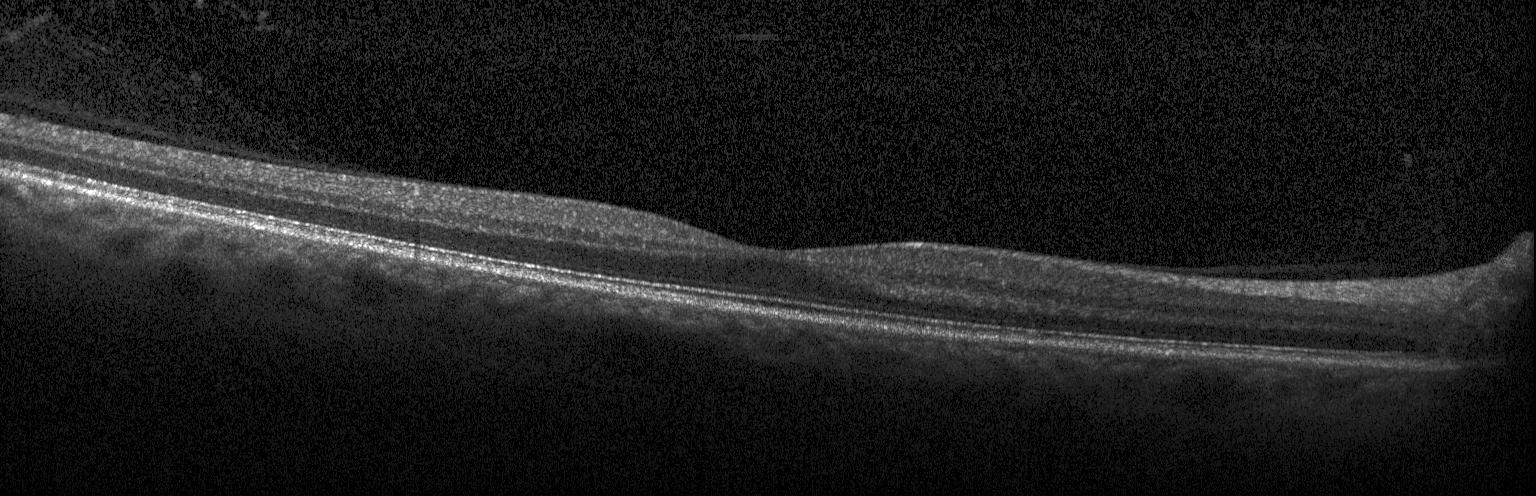

Spectral-domain OCT B-scan: no choroidal neovascularization, no diabetic macular edema, and no drusen.